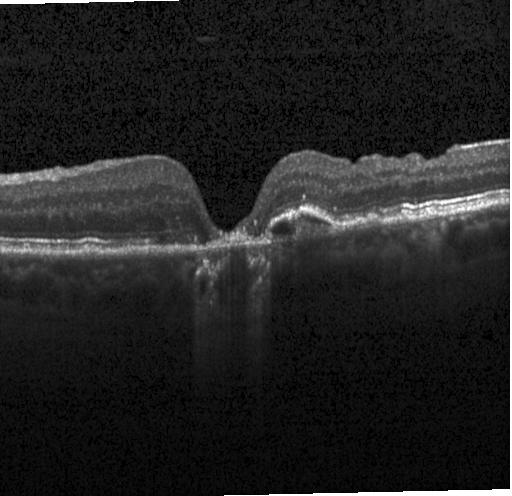 Dx: choroidal neovascularization (CNV).